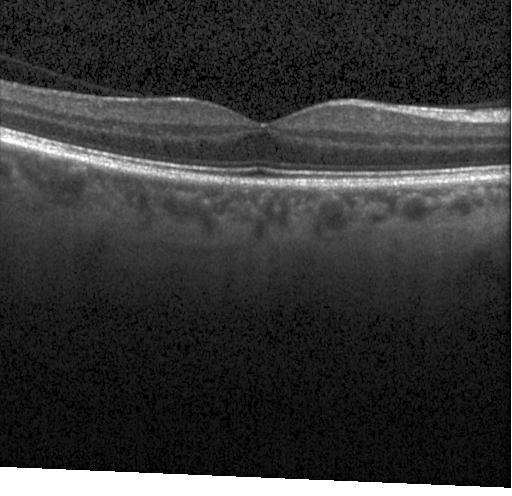

OCT B-scan showing no CNV, no DME, and no drusen.